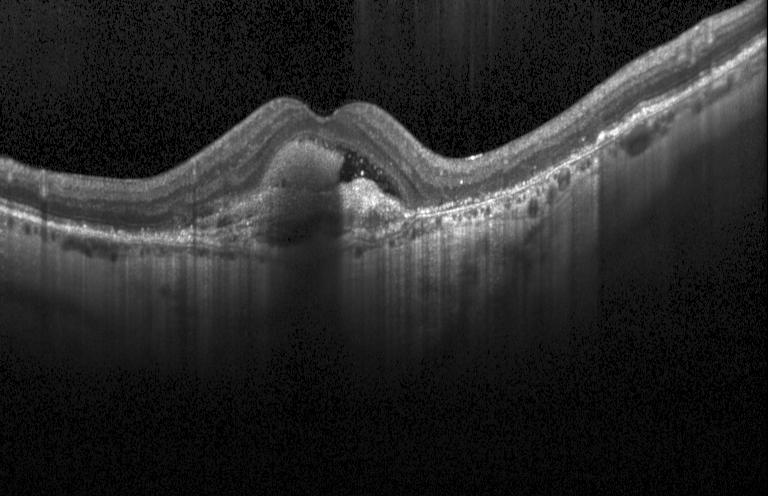

Spectral-domain OCT. Instrument: Heidelberg Spectralis. Macular scan. Optical coherence tomography scan — Finding: a choroidal neovascular membrane.